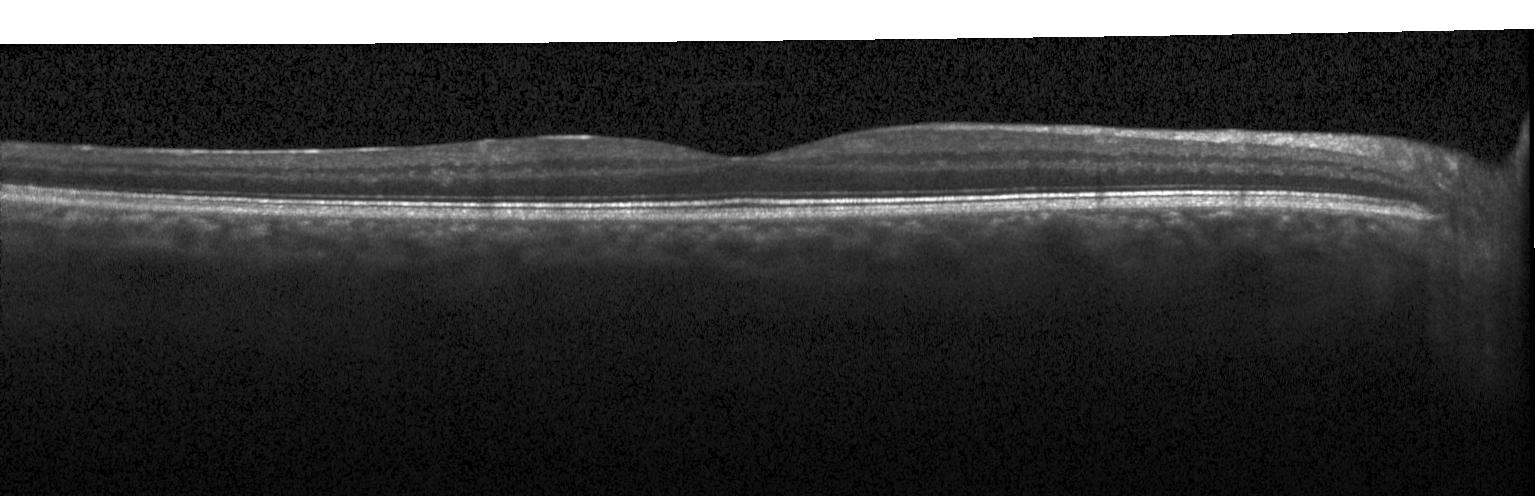 Dx: no choroidal neovascularization, diabetic macular edema, or drusen.